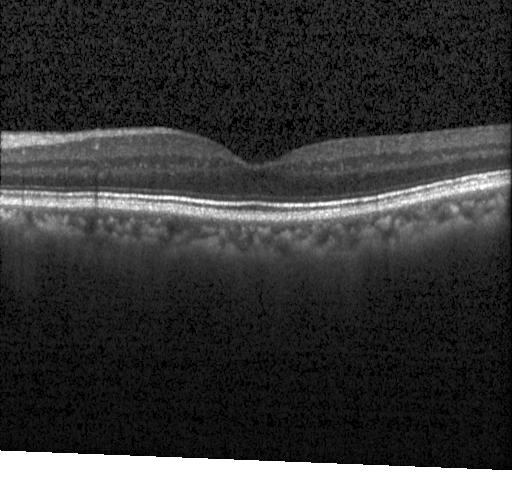
Retinal OCT cross-section. Finding: no CNV, no DME, and no drusen.